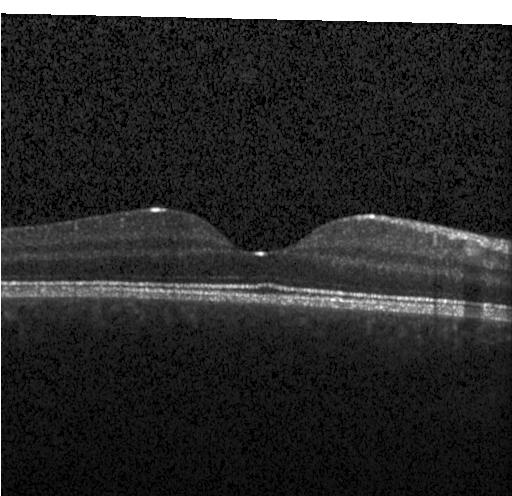 Impression: neither CNV, DME, nor drusen.